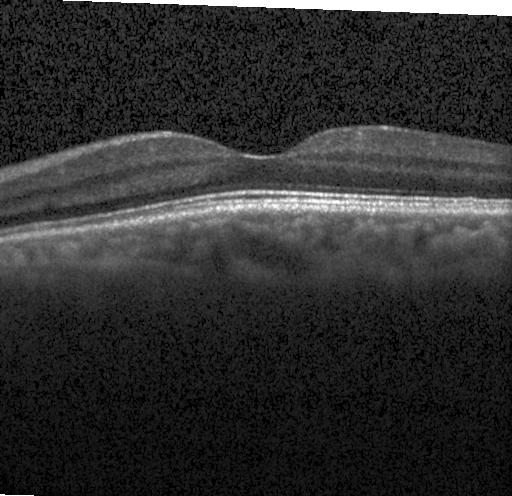

SD-OCT · optical coherence tomography B-scan. Assessment: neither choroidal neovascularization, diabetic macular edema, nor drusen.